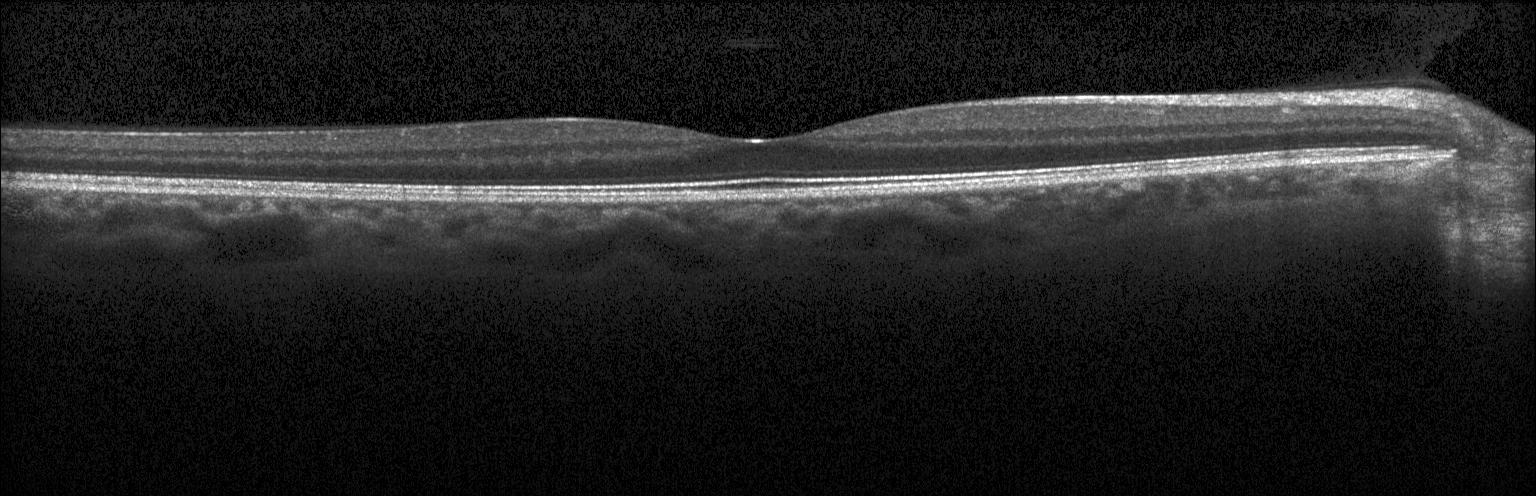
The scan shows neither choroidal neovascularization, diabetic macular edema, nor drusen.